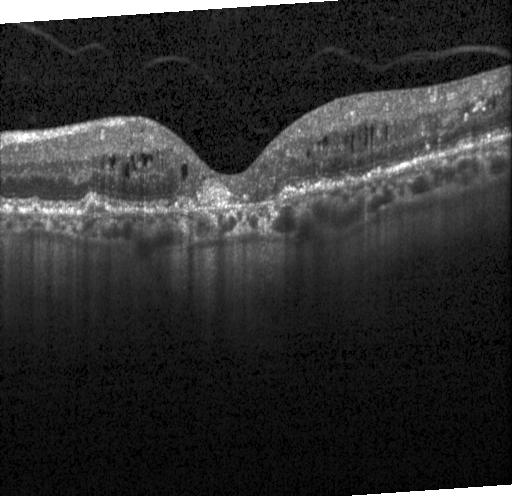

Assessment: CNV.